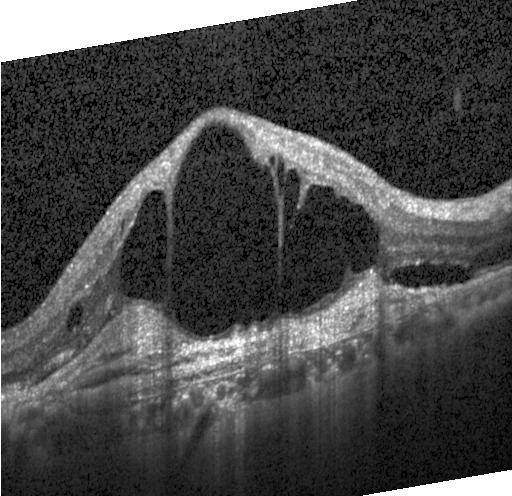
Dx: a choroidal neovascular membrane.